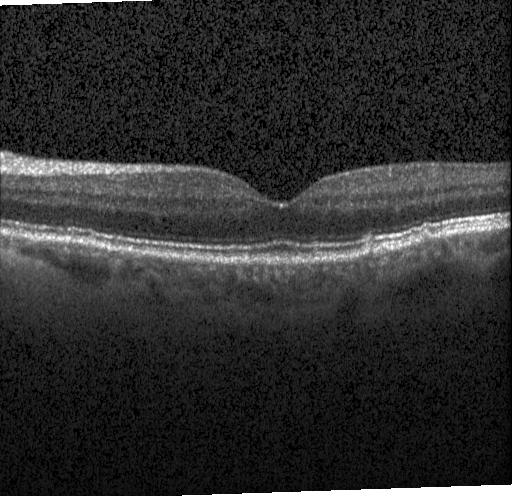
Fovea-centered; OCT B-scan
Diagnosis: drusen.